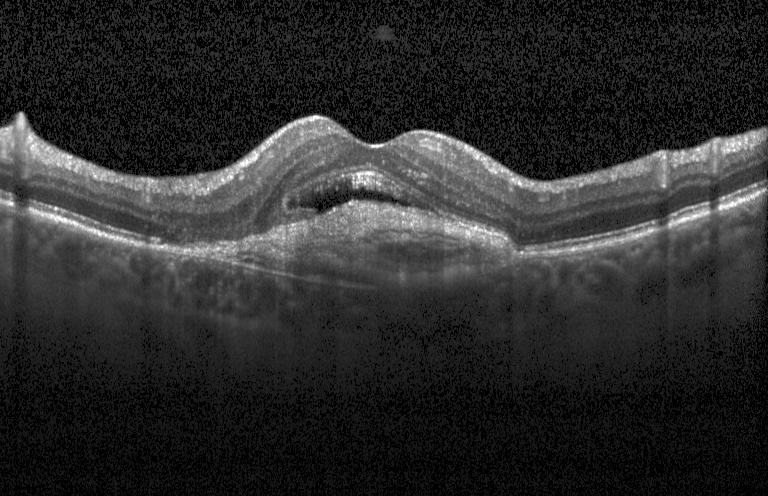
Diagnosis: choroidal neovascularization (CNV).